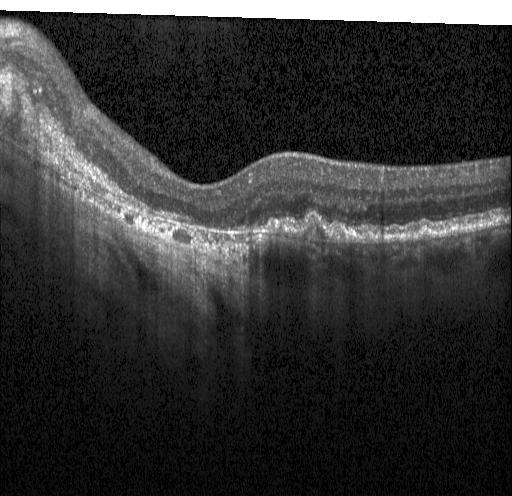

Retinal OCT cross-section — Choroidal neovascularization (CNV).